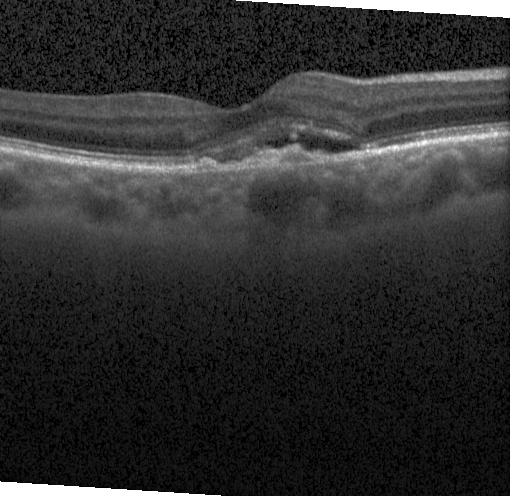 OCT B-scan — Impression: a choroidal neovascular membrane.